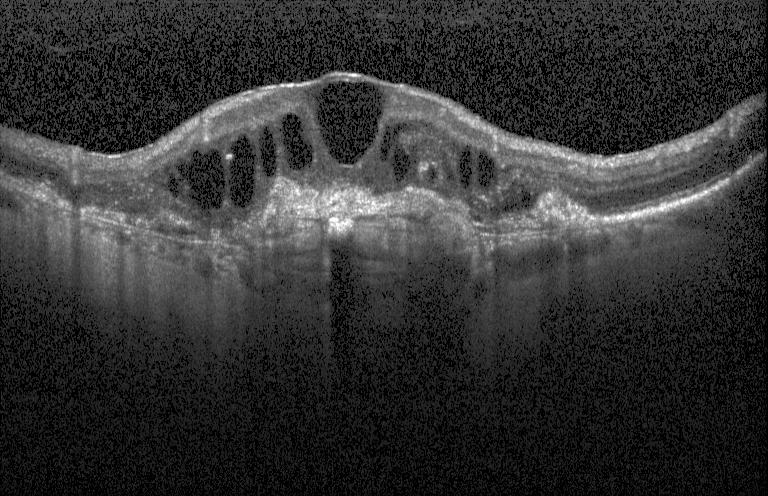

Spectral-domain OCT, acquired on a Heidelberg Spectralis, horizontal scan through the fovea, optical coherence tomography B-scan — Dx: a choroidal neovascular membrane.